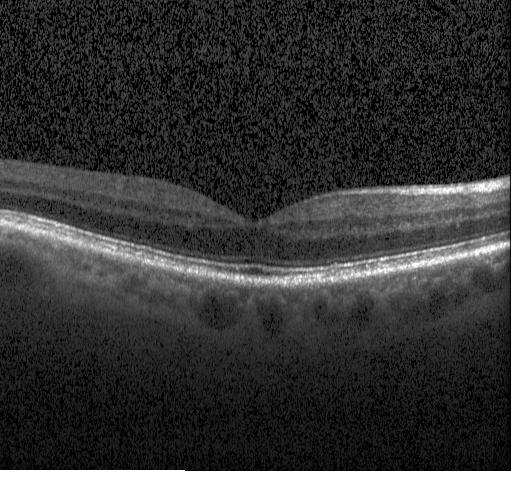

Retinal OCT cross-section · spectral-domain OCT — OCT finding: neither choroidal neovascularization, diabetic macular edema, nor drusen.